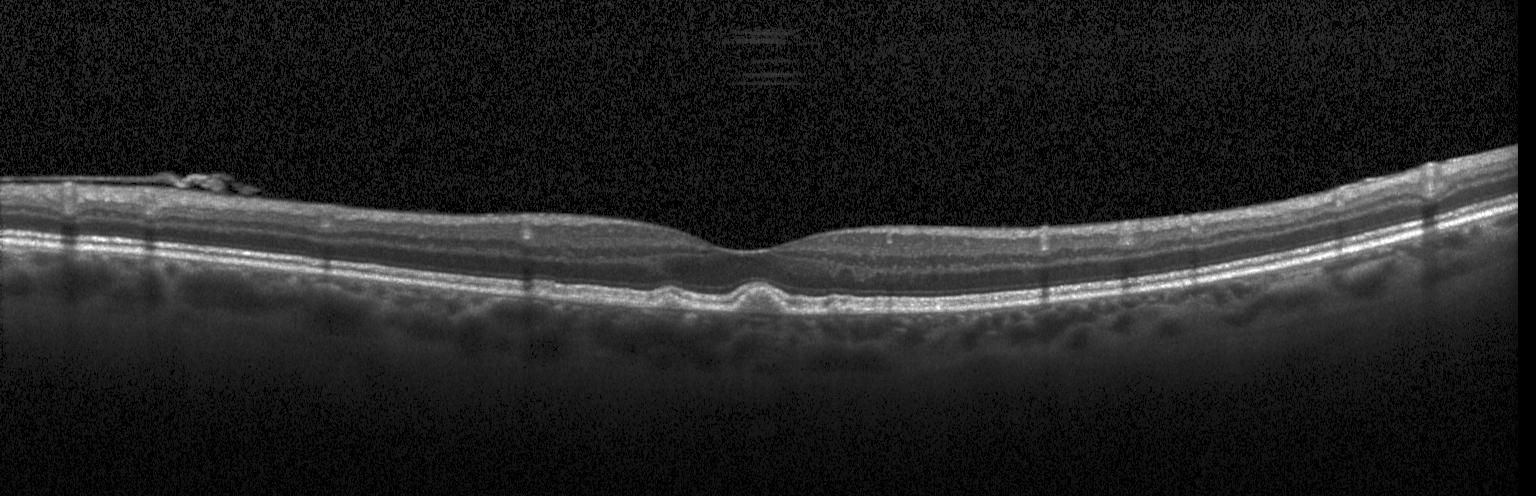
Spectral-domain OCT. Retinal OCT B-scan. Heidelberg Spectralis OCT system. Dx: multiple drusen.